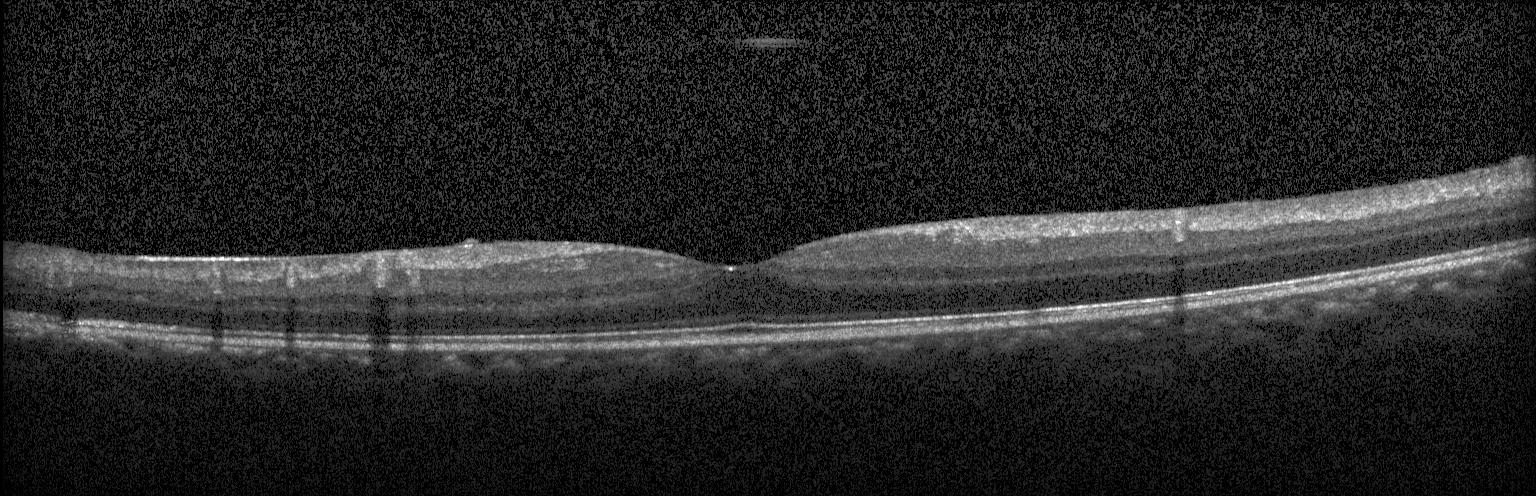

OCT B-scan — Dx: no choroidal neovascularization, diabetic macular edema, or drusen.